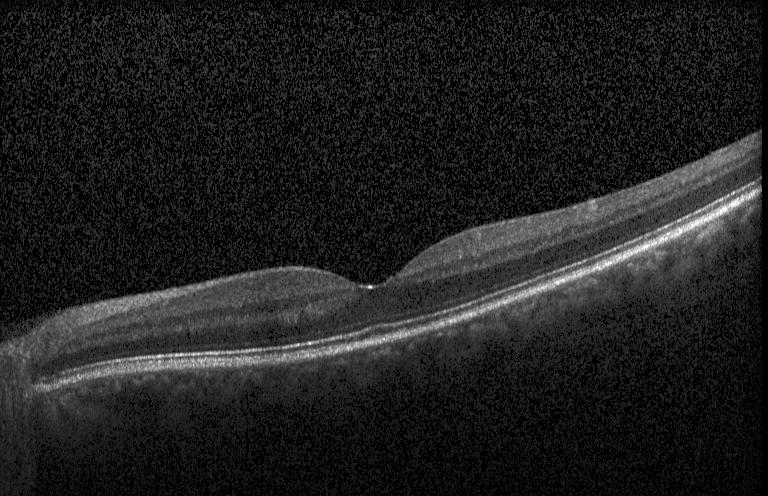
Diagnosis: no choroidal neovascularization, no diabetic macular edema, and no drusen.